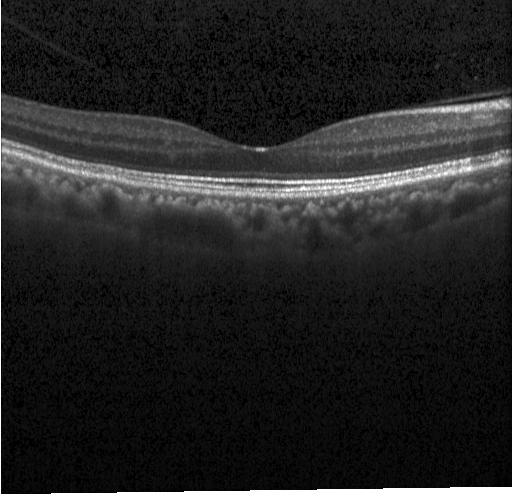 Through the macula; retinal OCT B-scan; spectral-domain optical coherence tomography; instrument: Heidelberg Spectralis
Impression: no CNV, DME, or drusen.